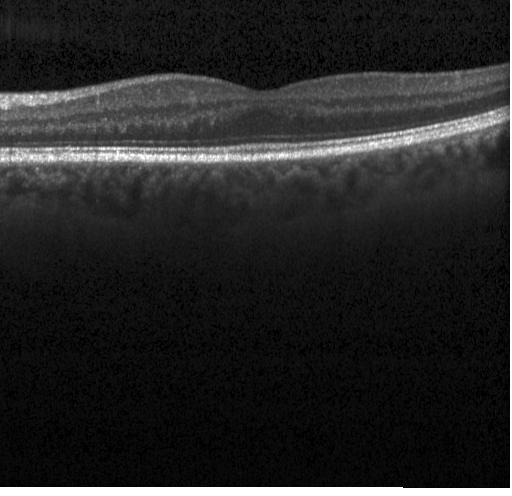

Centered on the fovea. Heidelberg Spectralis OCT system. Optical coherence tomography scan. Impression: neither CNV, DME, nor drusen.